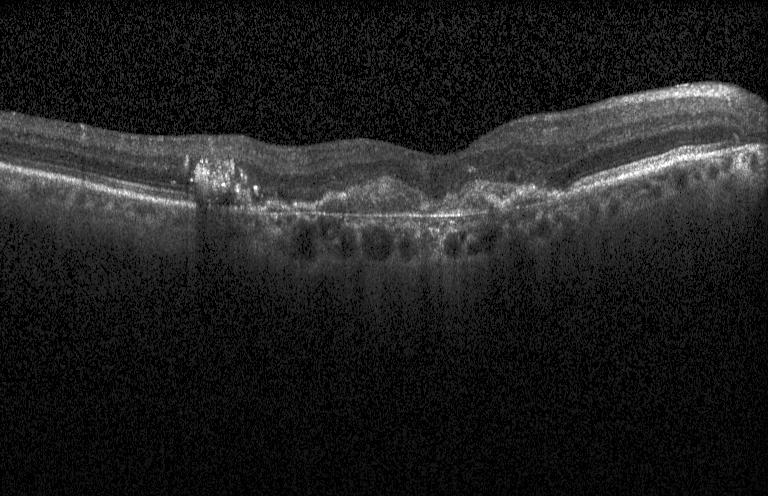
Spectral-domain optical coherence tomography · retinal OCT cross-section · Heidelberg Spectralis OCT system.
This B-scan demonstrates a choroidal neovascular membrane.